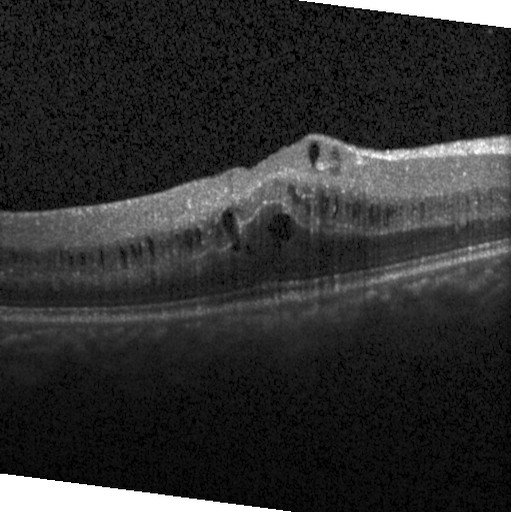 OCT line scan. SD-OCT. Diagnosis: diabetic macular edema (DME).